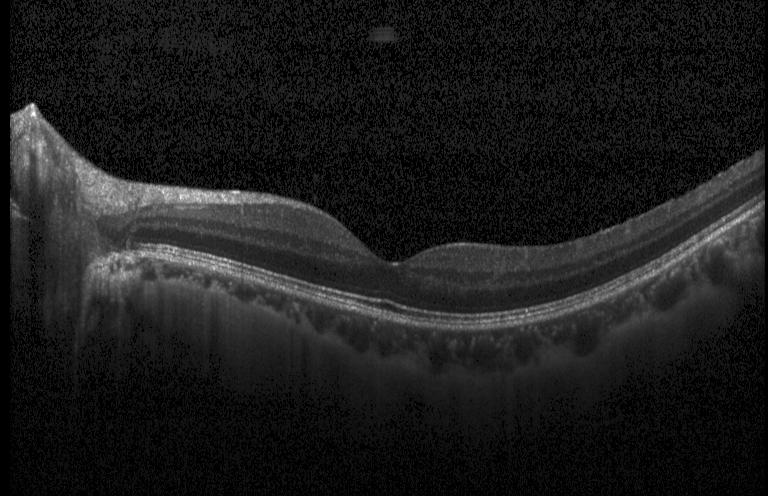

Heidelberg Spectralis OCT system; retinal OCT B-scan; spectral-domain OCT.
This B-scan demonstrates no choroidal neovascularization, diabetic macular edema, or drusen.